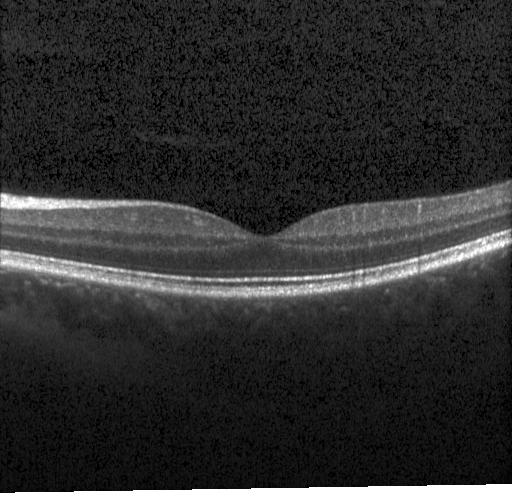 Retinal OCT B-scan · spectral-domain optical coherence tomography · macular scan
Macular OCT: no choroidal neovascularization, diabetic macular edema, or drusen.